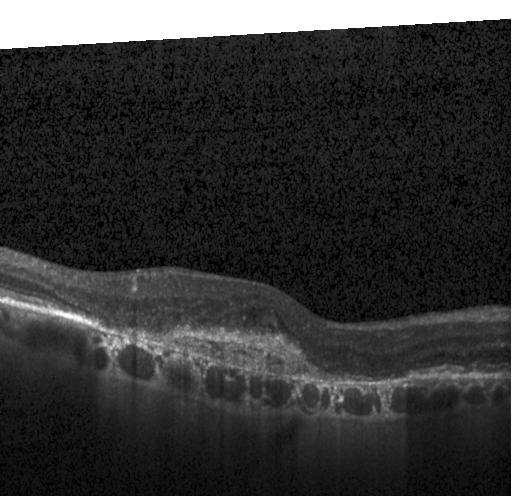 Acquired on a Heidelberg Spectralis. Centered on the fovea. Retinal OCT cross-section. Spectral-domain OCT — Diagnosis: a choroidal neovascular membrane.